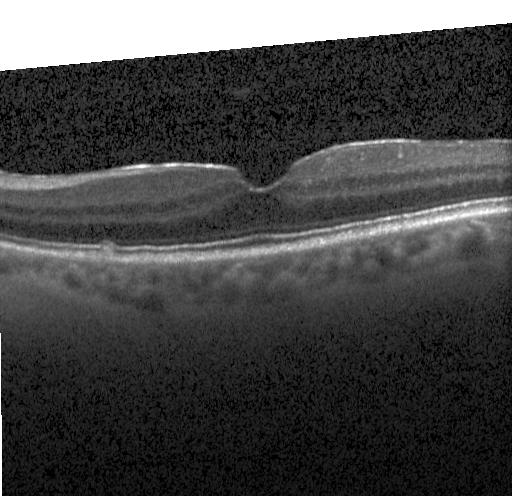

OCT line scan. This B-scan demonstrates sub-RPE drusenoid deposits.